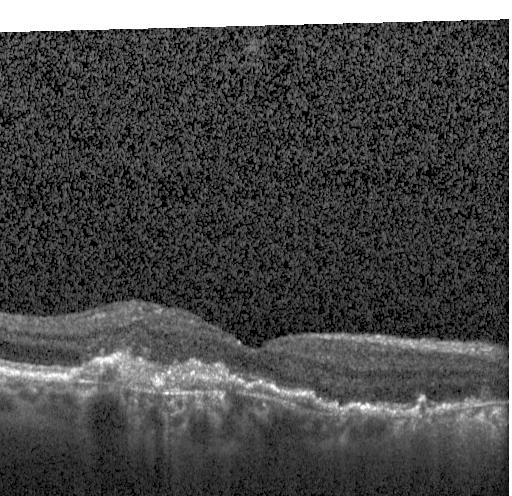 Dx: a choroidal neovascular membrane.